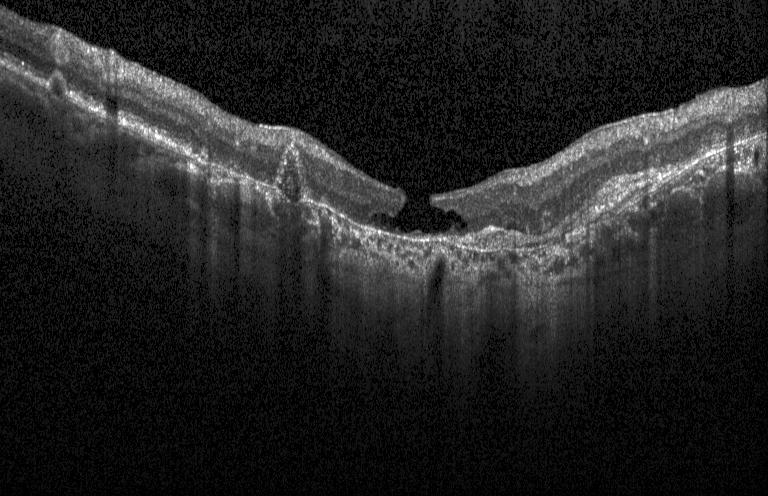 Instrument: Heidelberg Spectralis. Spectral-domain OCT. Optical coherence tomography B-scan. Fovea-centered
Finding: a choroidal neovascular membrane.